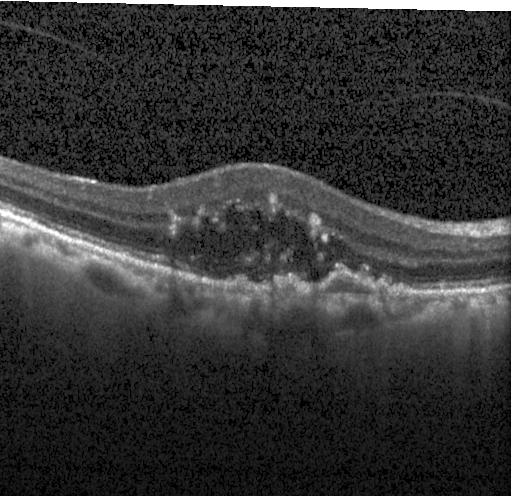
Dx: a choroidal neovascular membrane.